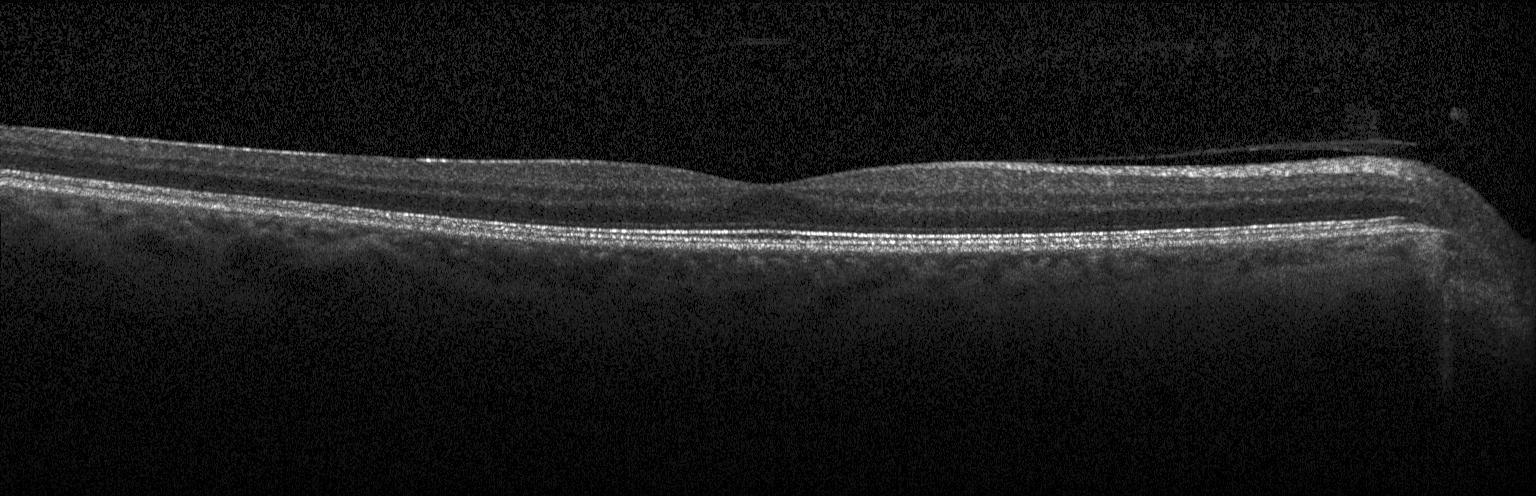 OCT line scan
Finding: no evidence of choroidal neovascularization, diabetic macular edema, or drusen.